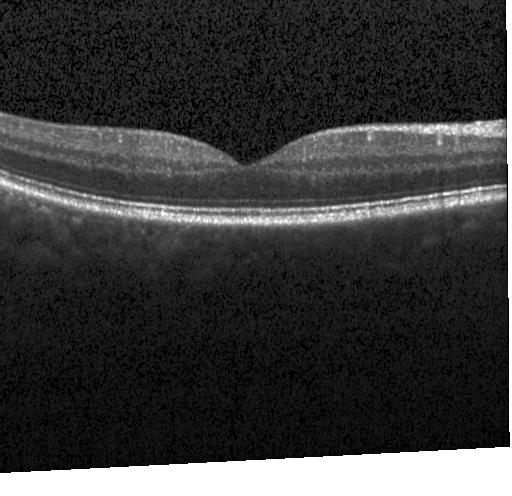

Optical coherence tomography scan.
Impression: no choroidal neovascularization, diabetic macular edema, or drusen.